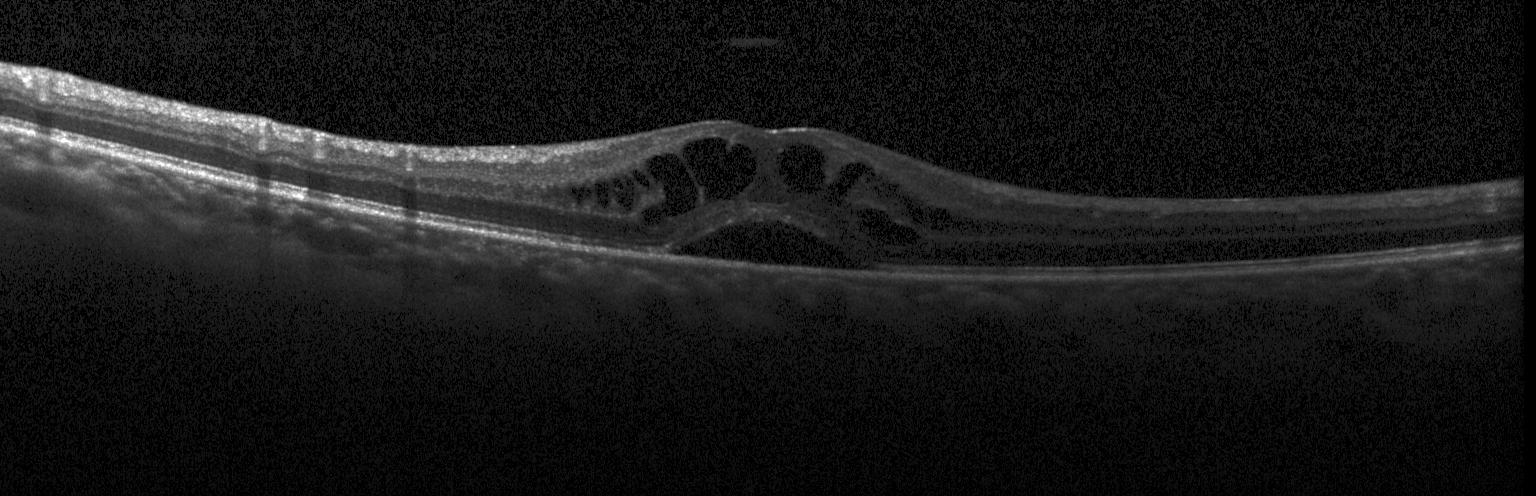

Macular OCT demonstrating diabetic macular edema (DME).